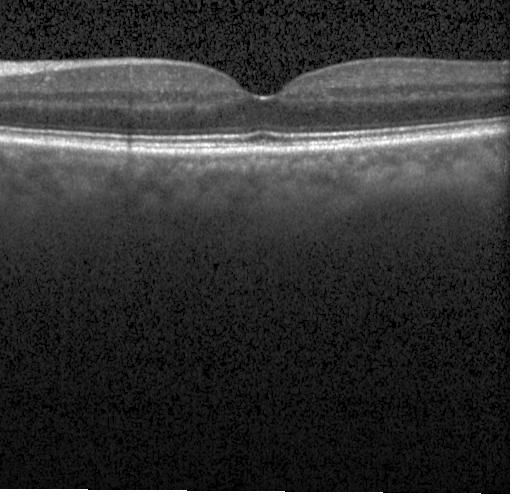

Impression: no CNV, no DME, and no drusen.